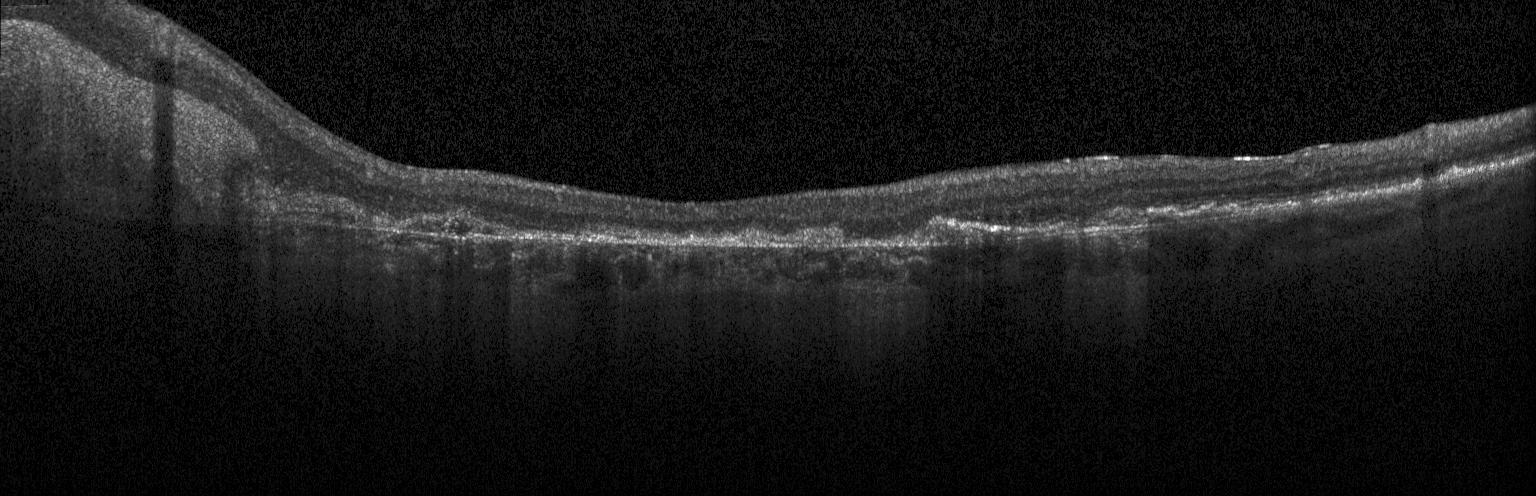

Retinal OCT B-scan — Impression: a choroidal neovascular membrane.